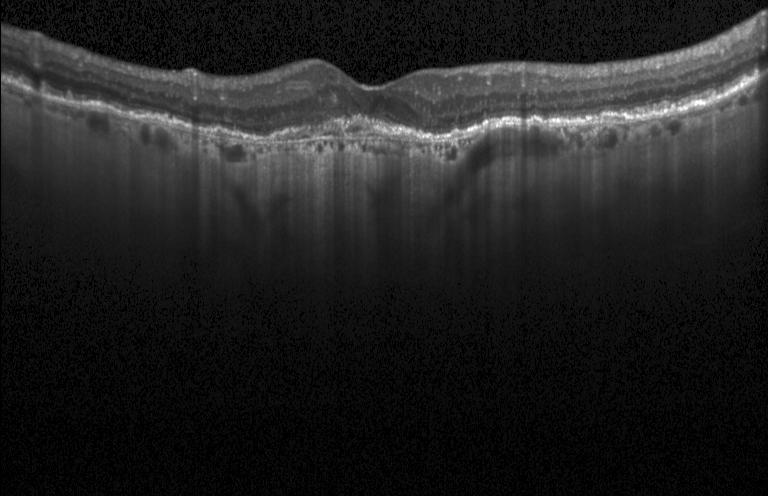
Impression: a choroidal neovascular membrane.